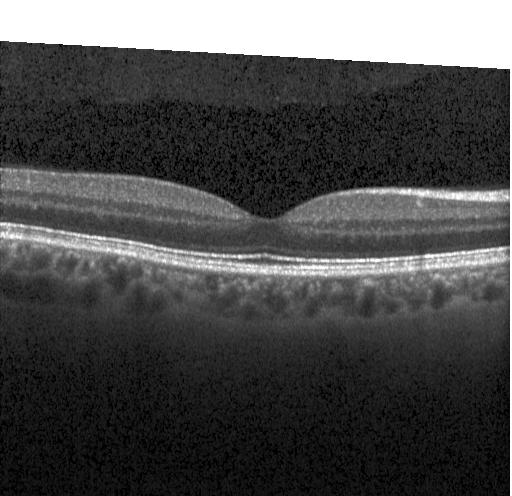 SD-OCT · retinal OCT B-scan. Impression: no choroidal neovascularization, no diabetic macular edema, and no drusen.